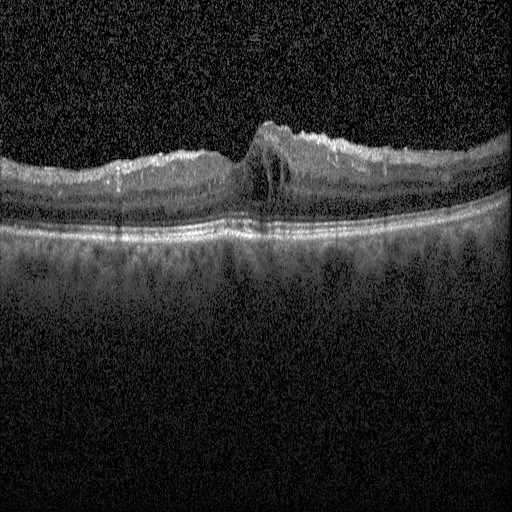

Retinal OCT cross-section showing DME.